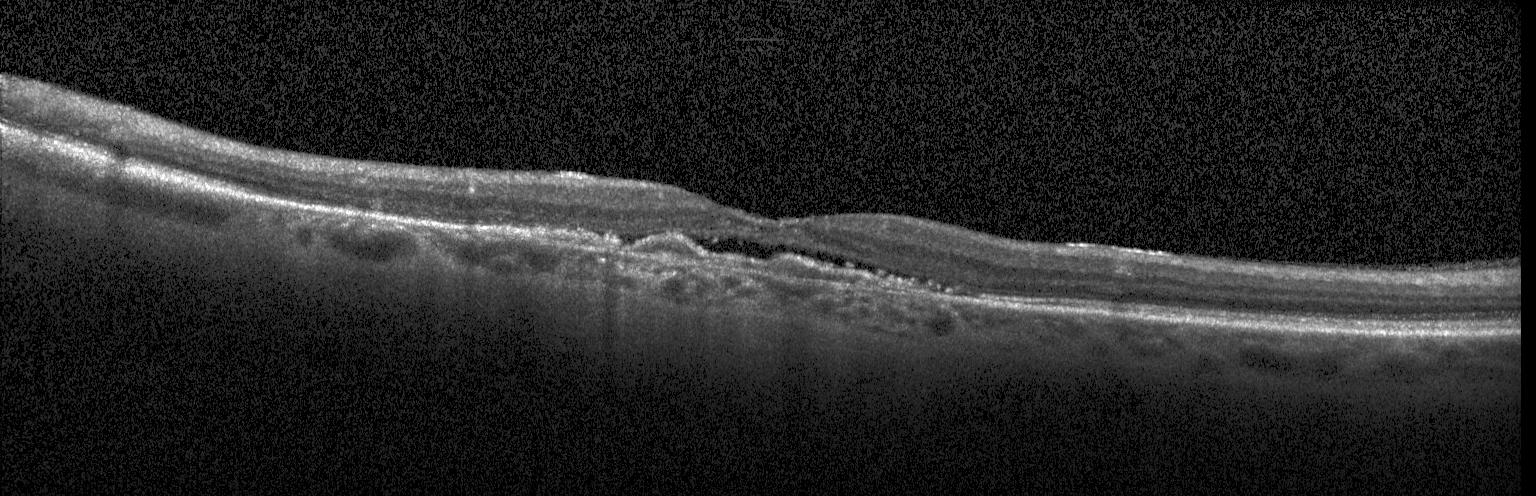
OCT scan showing a choroidal neovascular membrane.